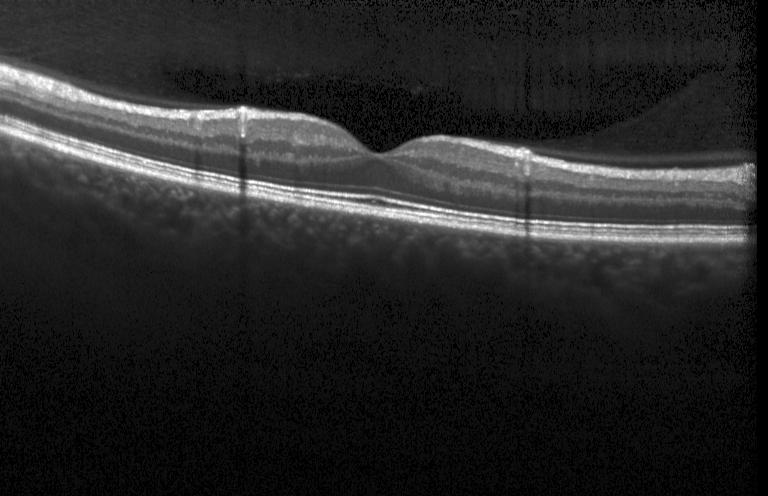
Retinal OCT B-scan
Assessment: neither choroidal neovascularization, diabetic macular edema, nor drusen.